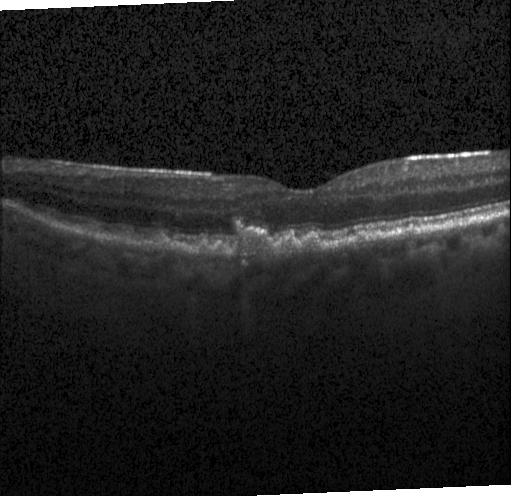 Diagnosis: choroidal neovascularization (CNV).